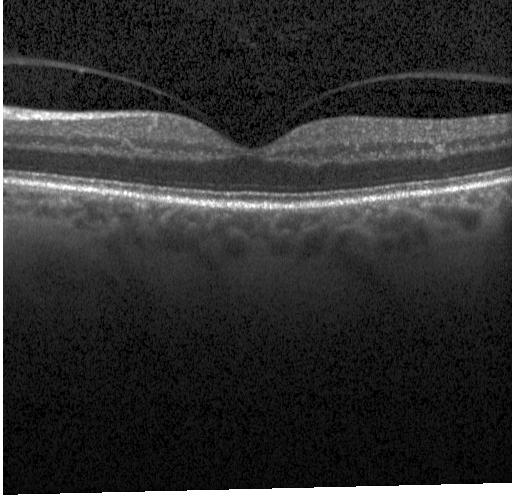

Macular OCT: no evidence of choroidal neovascularization, diabetic macular edema, or drusen.